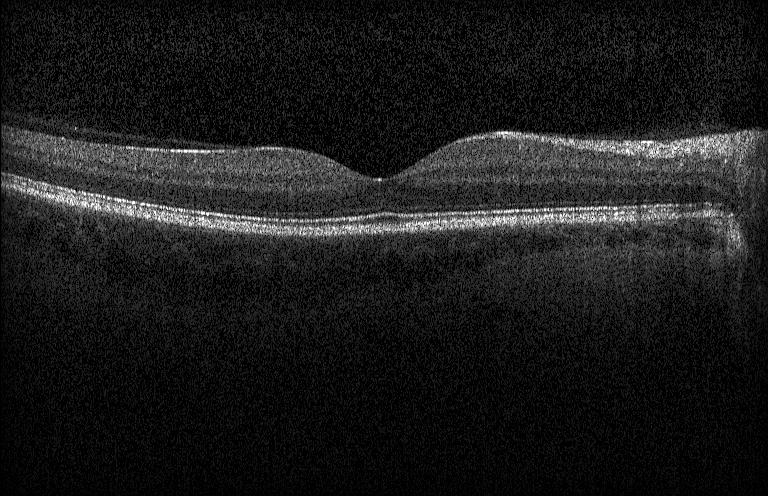 Retinal OCT cross-section.
Macular OCT: no evidence of CNV, DME, or drusen.